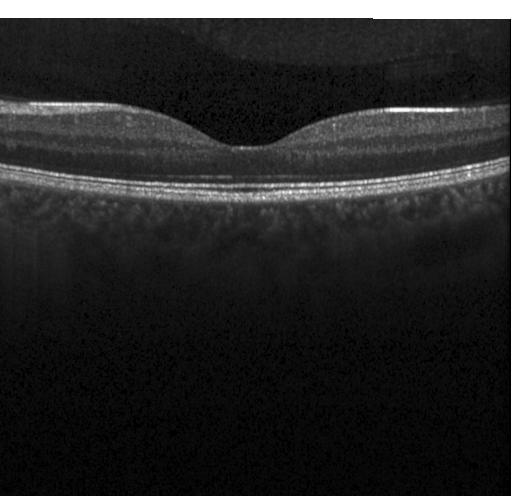

Through the macula; spectral-domain optical coherence tomography; OCT B-scan; acquired on a Heidelberg Spectralis.
Dx: no CNV, no DME, and no drusen.